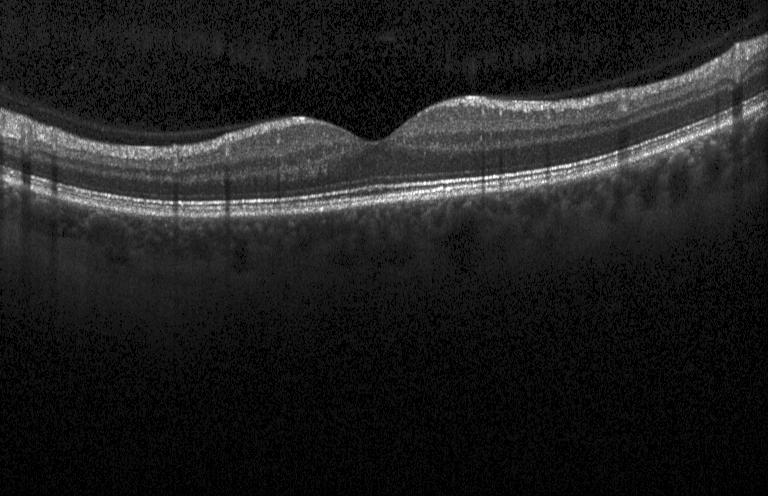 Acquired on a Heidelberg Spectralis, retinal OCT cross-section
Finding: no evidence of choroidal neovascularization, diabetic macular edema, or drusen.